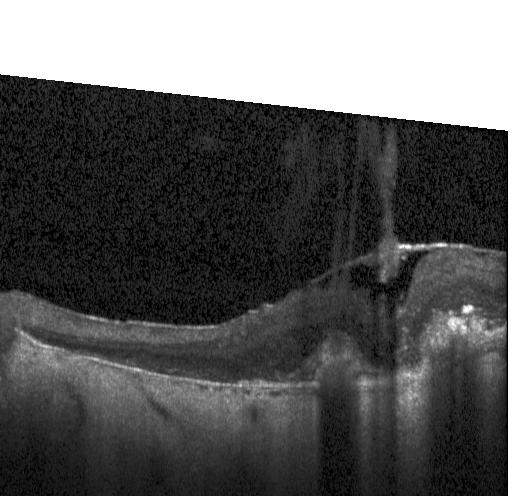 Diagnosis: CNV.